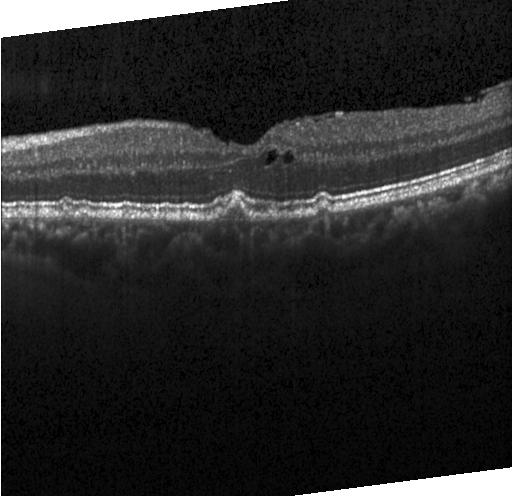 SD-OCT. OCT B-scan. Instrument: Heidelberg Spectralis
OCT finding: drusen.